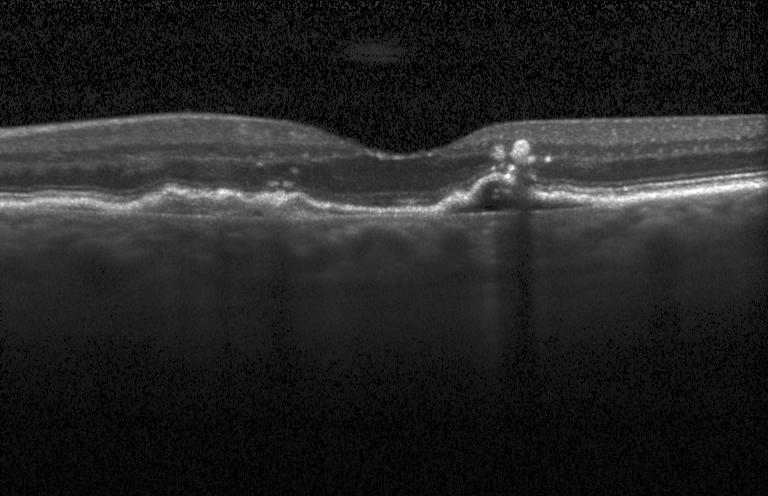
Optical coherence tomography scan; instrument: Heidelberg Spectralis; SD-OCT; macular scan
This B-scan demonstrates a choroidal neovascular membrane.